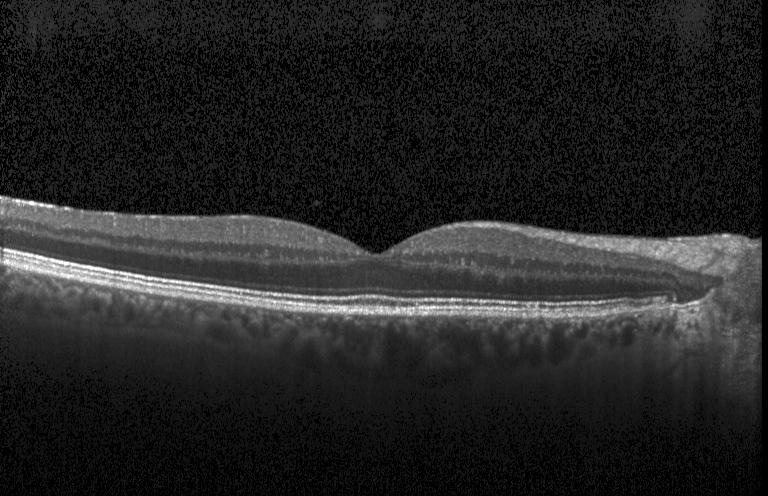 Macular scan · optical coherence tomography scan.
This B-scan demonstrates no CNV, DME, or drusen.